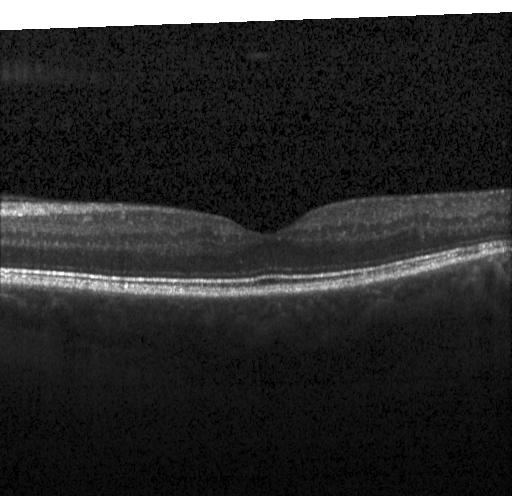 Instrument: Heidelberg Spectralis · horizontal scan through the fovea · OCT line scan · spectral-domain OCT.
Diagnosis: no CNV, no DME, and no drusen.